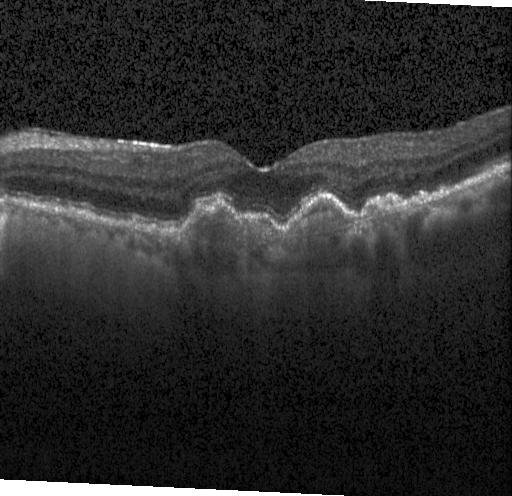
Dx: a choroidal neovascular membrane.